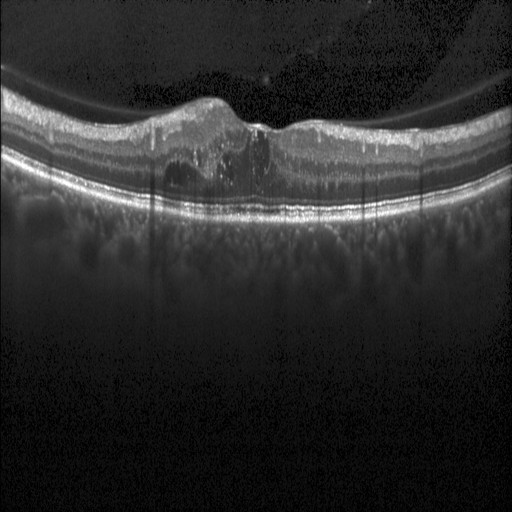

Diagnosis: diabetic macular edema.